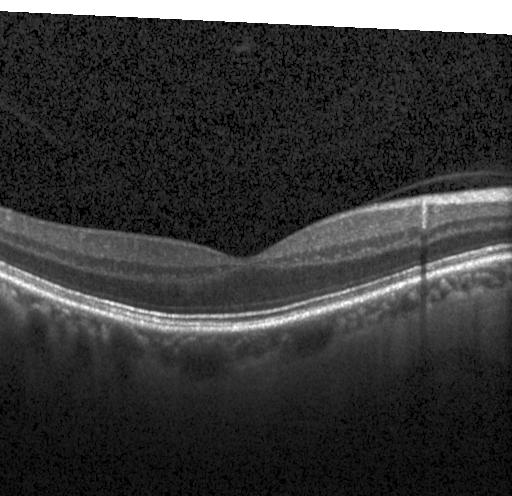 OCT line scan — Dx: no choroidal neovascularization, no diabetic macular edema, and no drusen.